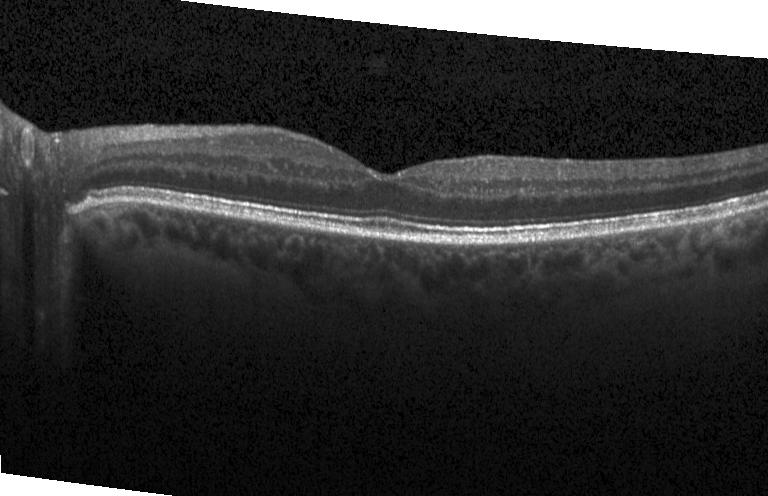 Diagnosis: no evidence of CNV, DME, or drusen.